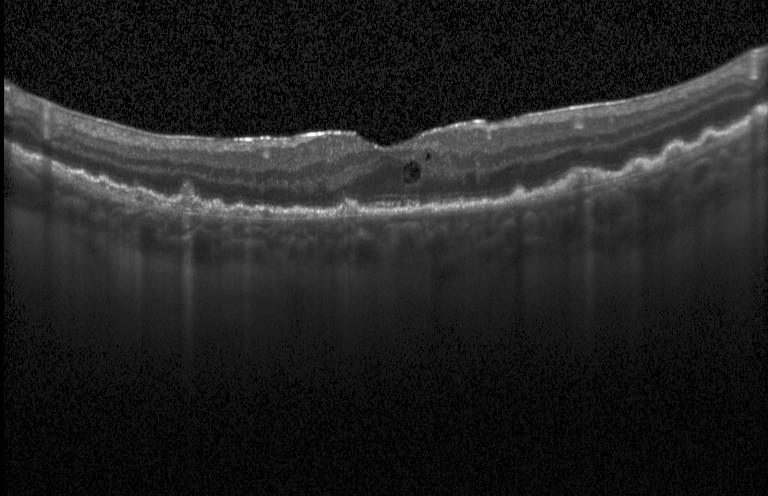 Dx: a choroidal neovascular membrane.